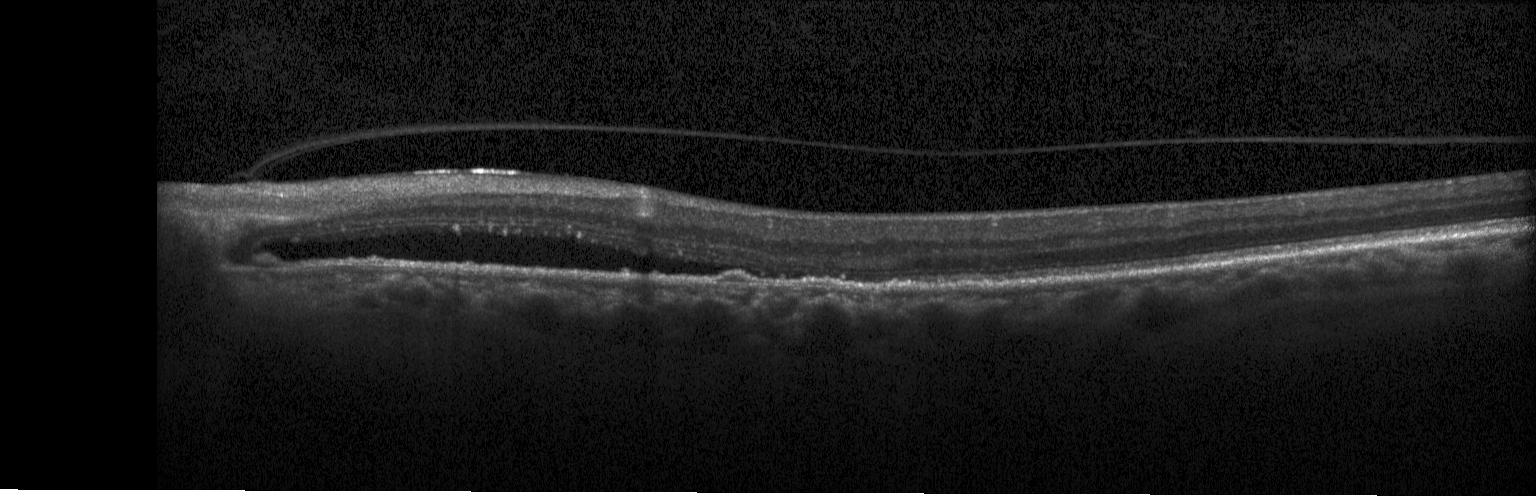 Macular OCT: a choroidal neovascular membrane.